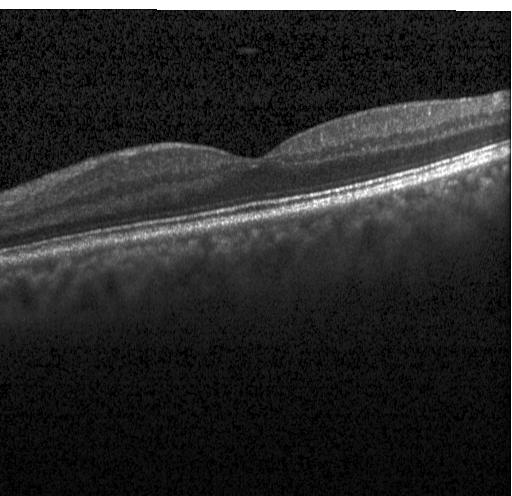
Optical coherence tomography scan
Impression: no CNV, no DME, and no drusen.